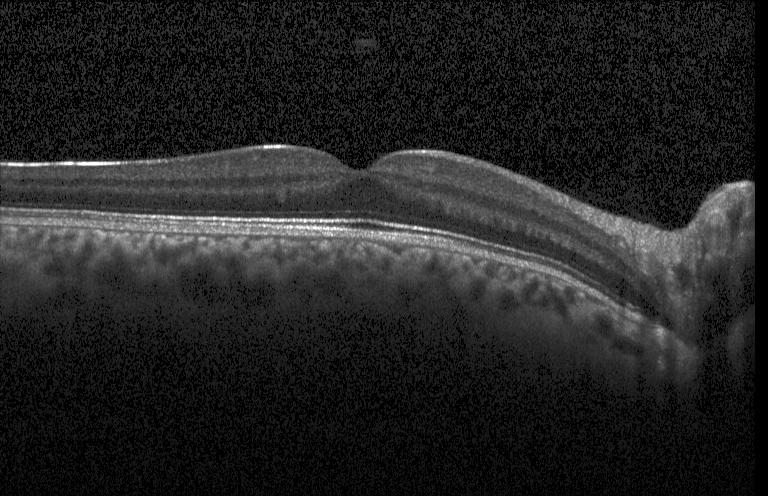
Heidelberg Spectralis, optical coherence tomography B-scan, spectral-domain OCT. Macular OCT: no CNV, DME, or drusen.